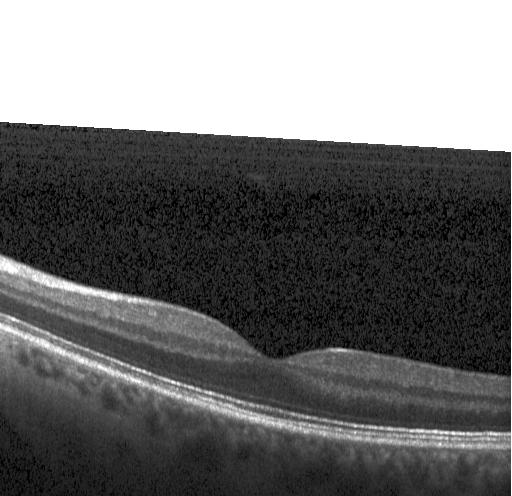

Dx: no evidence of CNV, DME, or drusen.